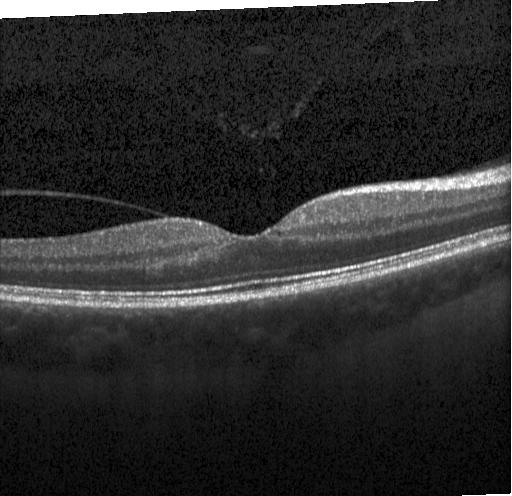
Impression: neither CNV, DME, nor drusen.